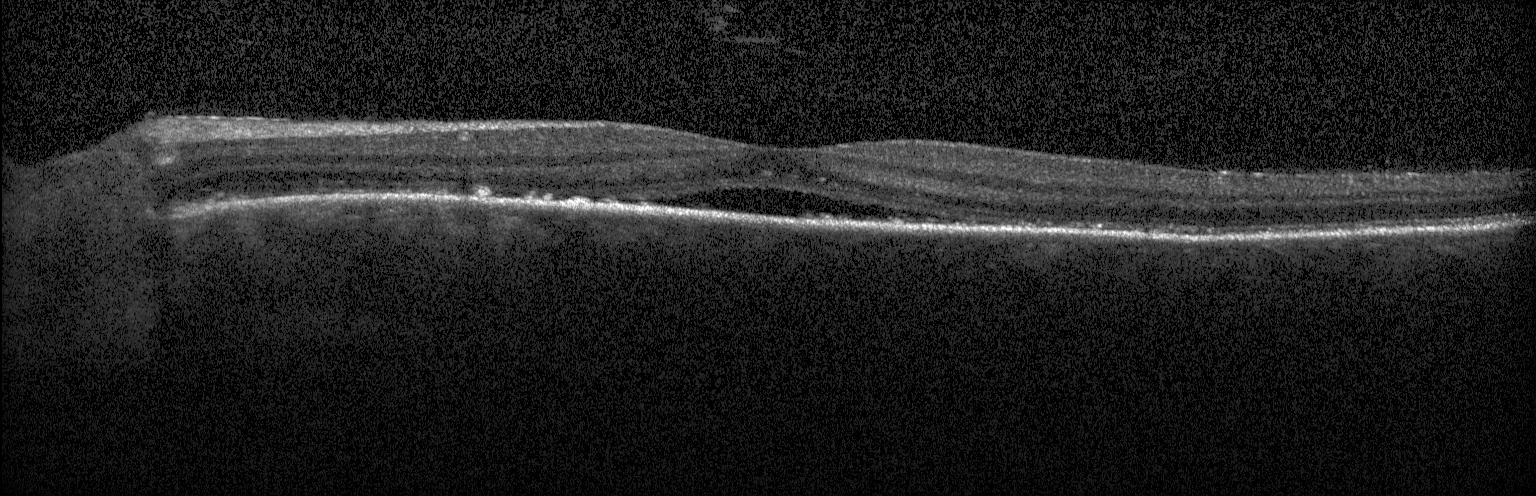

A choroidal neovascular membrane.